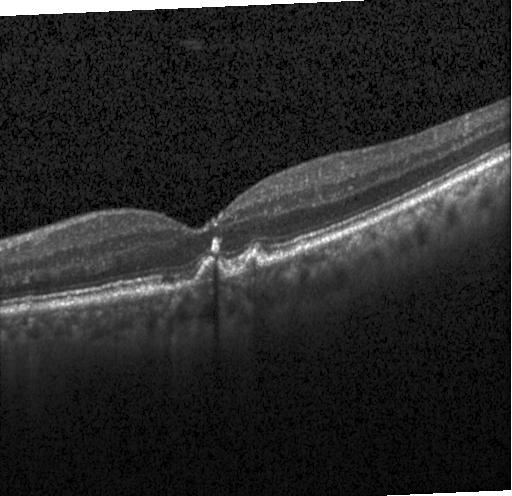 Optical coherence tomography B-scan · through the macula · Heidelberg Spectralis. Finding: sub-RPE drusenoid deposits.